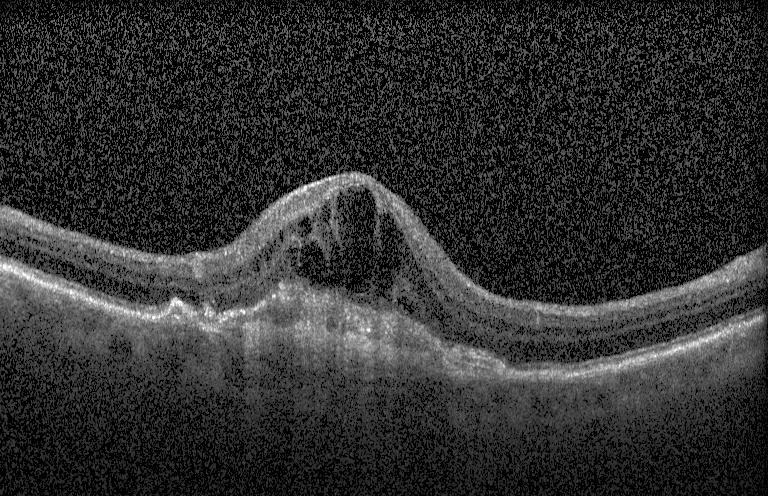 Diagnosis: choroidal neovascularization (CNV).